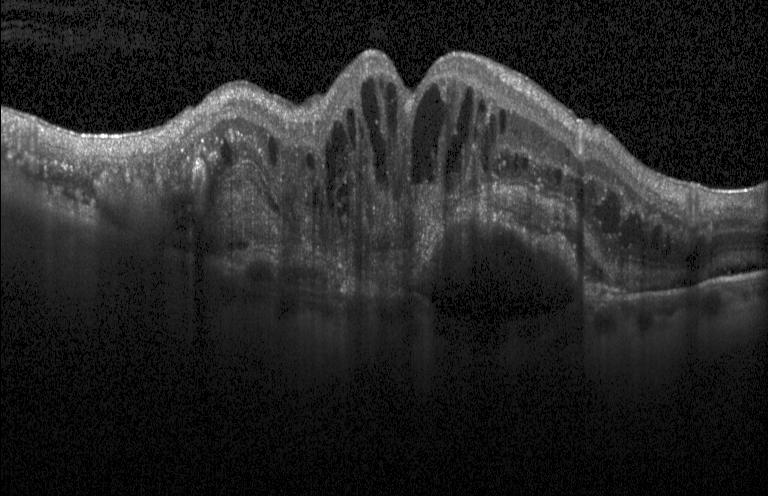 Impression: a choroidal neovascular membrane.